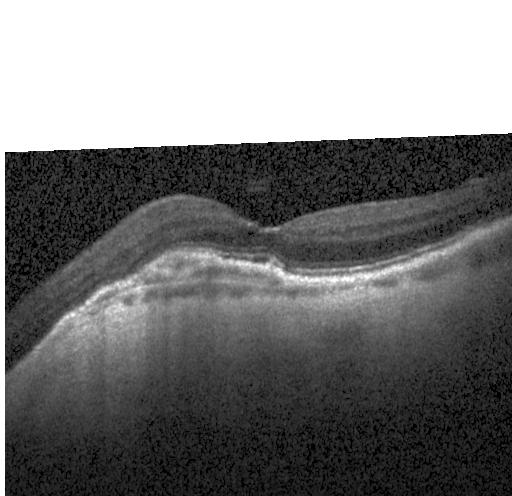 Spectral-domain OCT B-scan: a choroidal neovascular membrane.